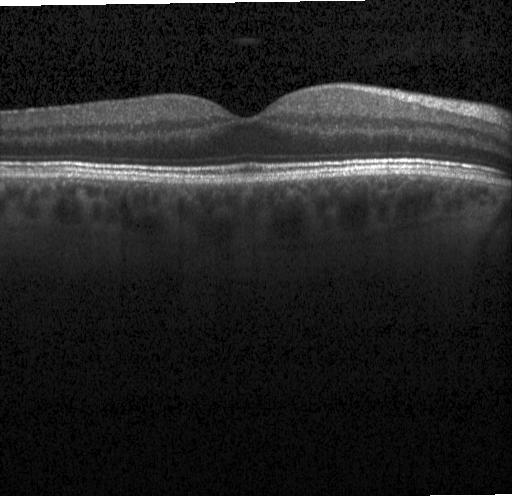

Retinal OCT B-scan. Impression: no choroidal neovascularization, no diabetic macular edema, and no drusen.